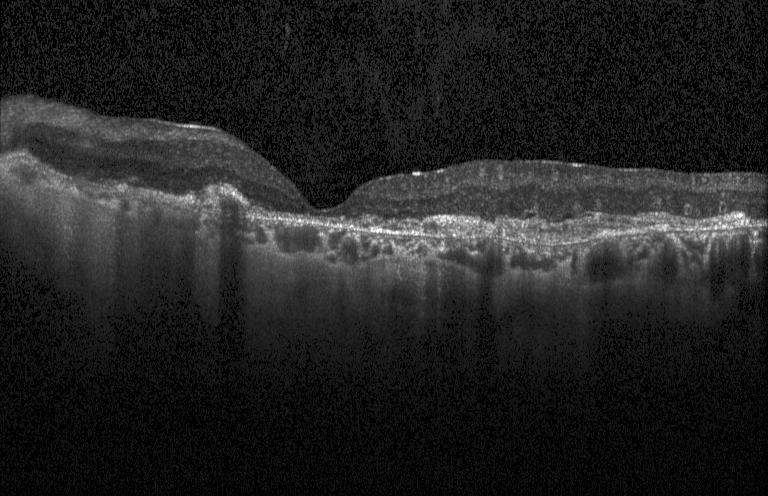 Finding: a choroidal neovascular membrane.